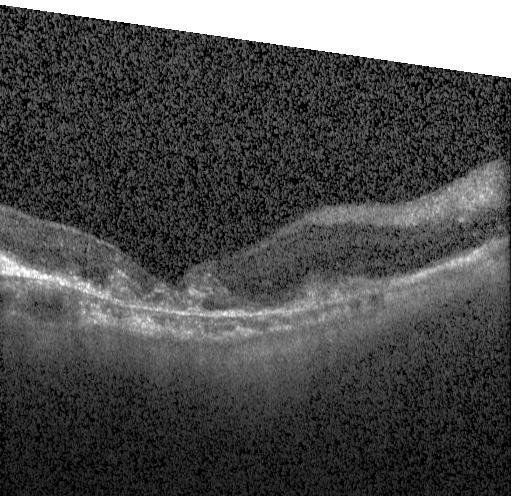
SD-OCT; horizontal scan through the fovea; instrument: Heidelberg Spectralis; retinal OCT B-scan
Dx: choroidal neovascularization.